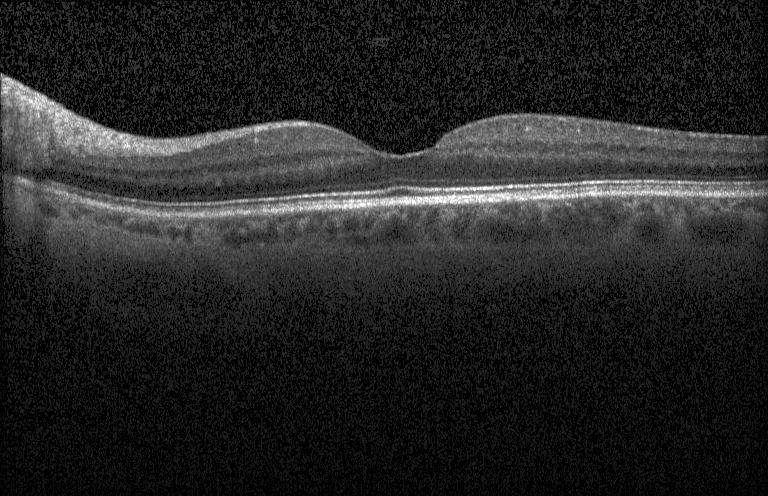 Horizontal scan through the fovea; acquired on a Heidelberg Spectralis; optical coherence tomography B-scan
Finding: no evidence of choroidal neovascularization, diabetic macular edema, or drusen.